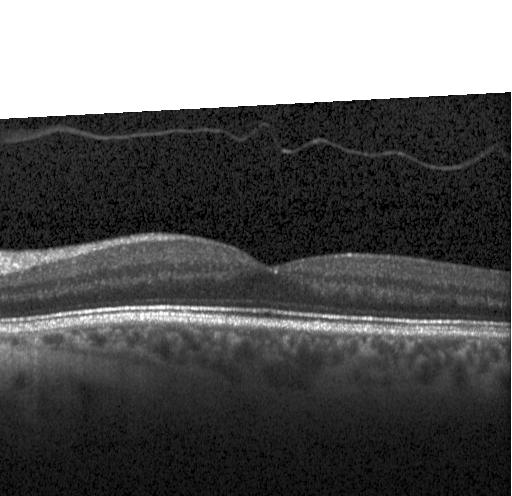

OCT B-scan
This B-scan demonstrates neither choroidal neovascularization, diabetic macular edema, nor drusen.